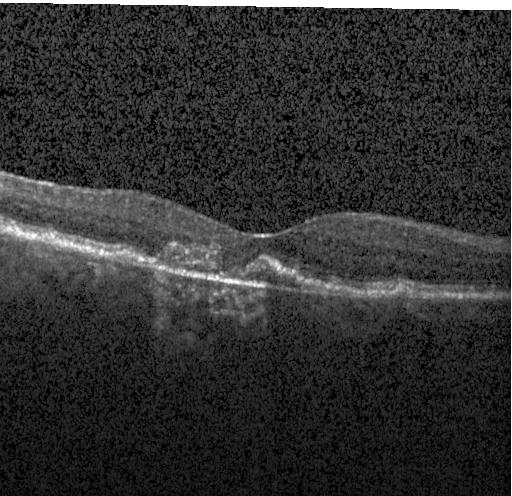

OCT scan showing a choroidal neovascular membrane.